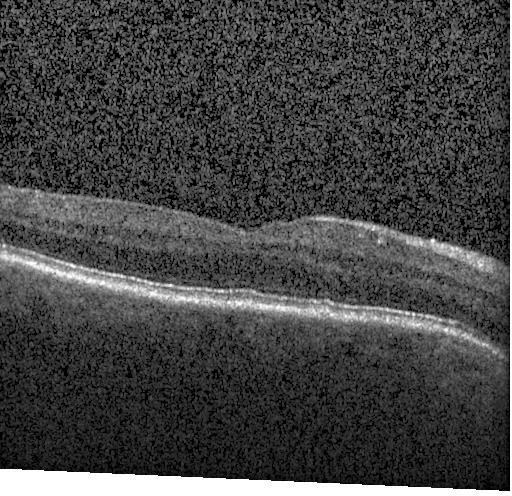
Acquired on a Heidelberg Spectralis · through the macula · OCT B-scan.
OCT finding: neither CNV, DME, nor drusen.